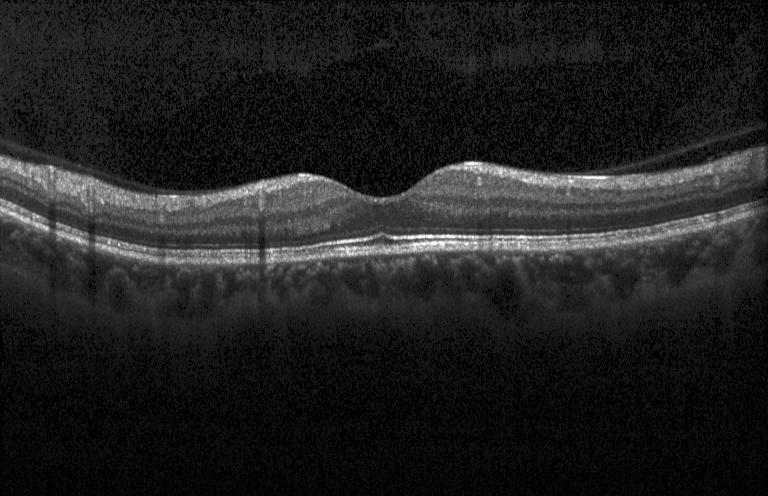

This B-scan demonstrates no CNV, no DME, and no drusen.